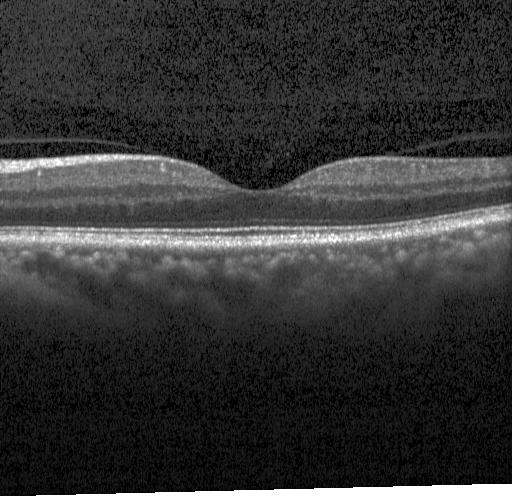
Retinal OCT B-scan, macular scan.
OCT finding: no CNV, DME, or drusen.